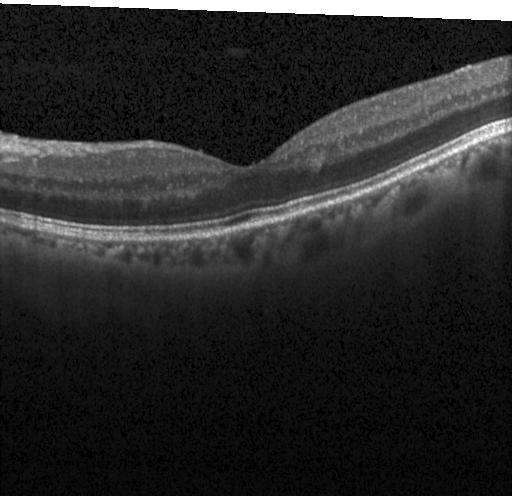
Diagnosis: neither choroidal neovascularization, diabetic macular edema, nor drusen.